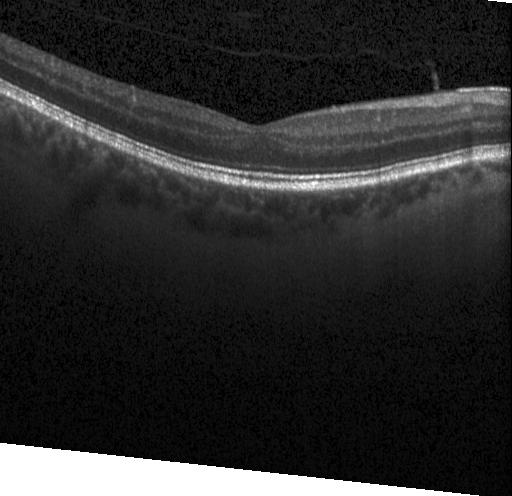 OCT B-scan showing no CNV, DME, or drusen.